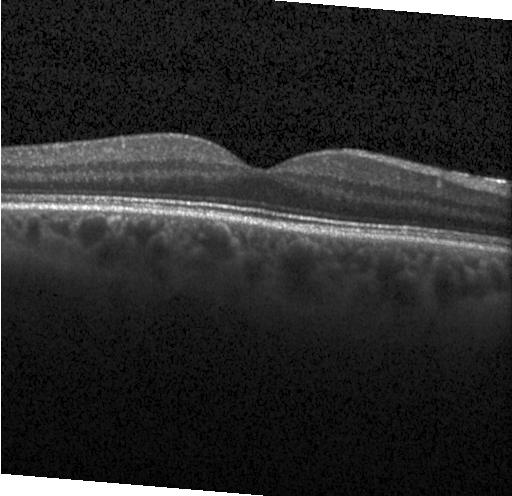 Fovea-centered. SD-OCT. OCT line scan.
Assessment: no CNV, DME, or drusen.